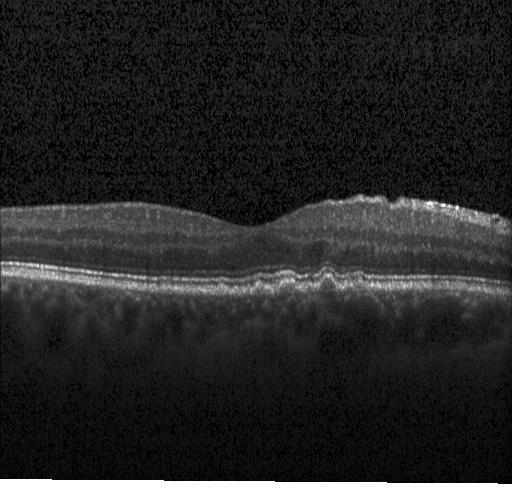 OCT B-scan, instrument: Heidelberg Spectralis.
Dx: sub-RPE drusenoid deposits.